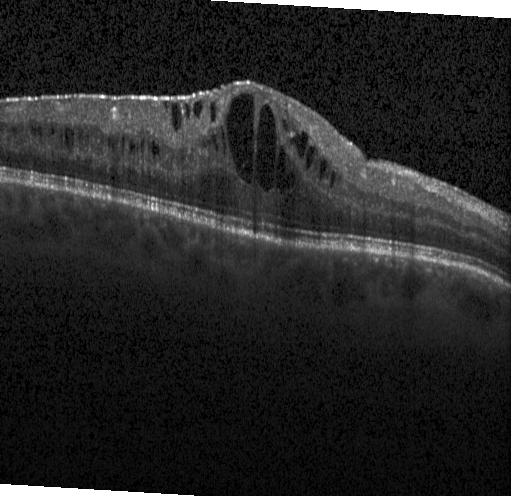
OCT line scan. Macular OCT: DME.